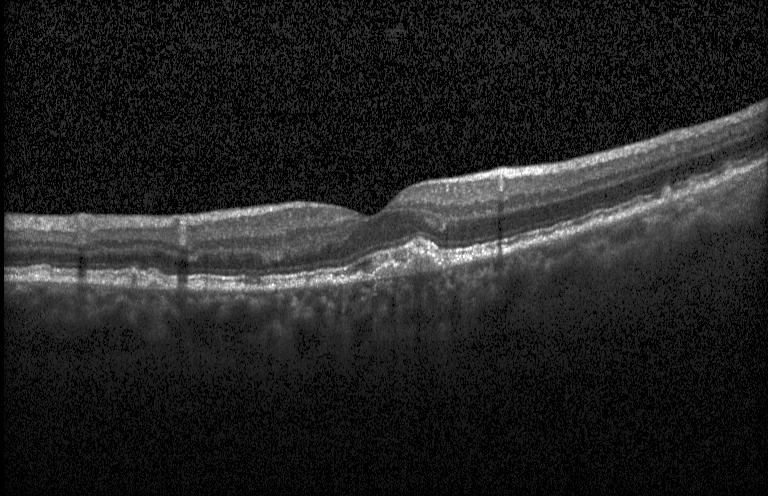
OCT B-scan; fovea-centered.
Diagnosis: multiple drusen.